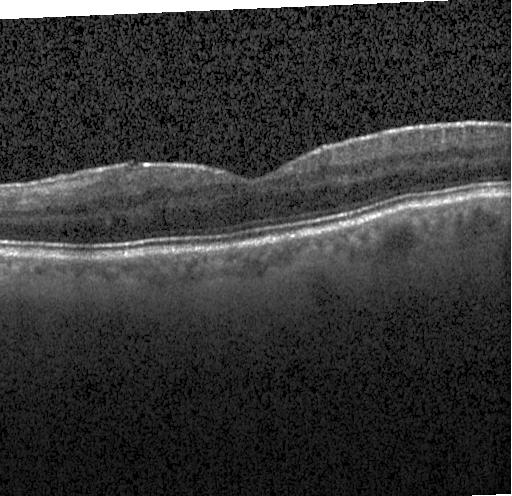

Optical coherence tomography B-scan, Heidelberg Spectralis.
Finding: no CNV, DME, or drusen.